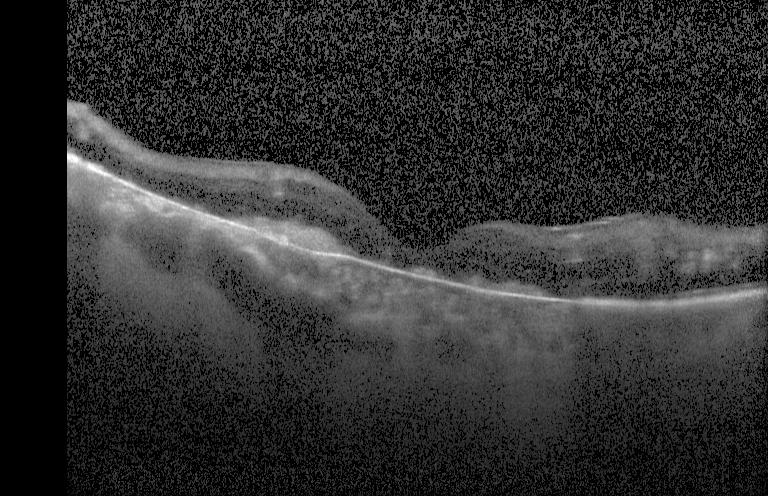 Optical coherence tomography B-scan; spectral-domain optical coherence tomography; Heidelberg Spectralis
Finding: CNV.